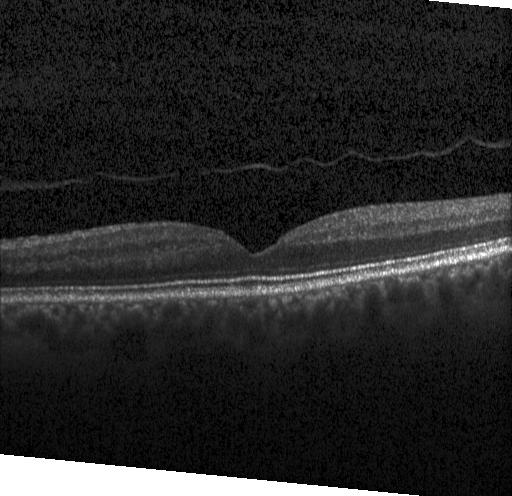

Retinal OCT cross-section showing no CNV, DME, or drusen.